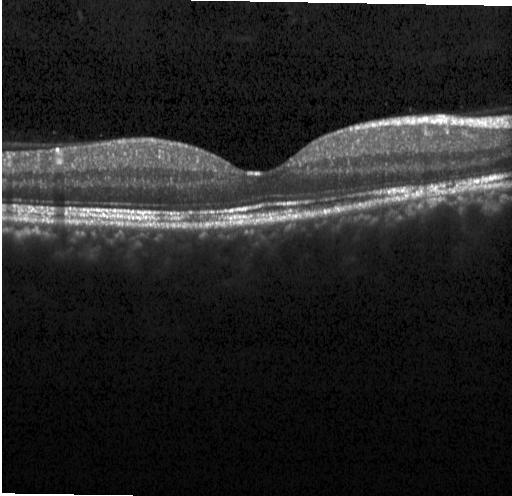 Spectral-domain OCT B-scan: no choroidal neovascularization, no diabetic macular edema, and no drusen.